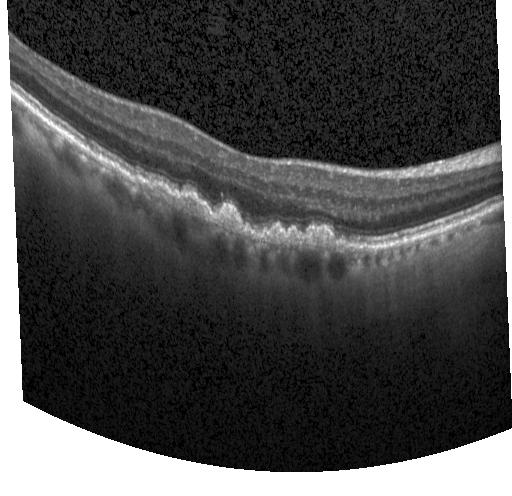
Impression: multiple drusen.